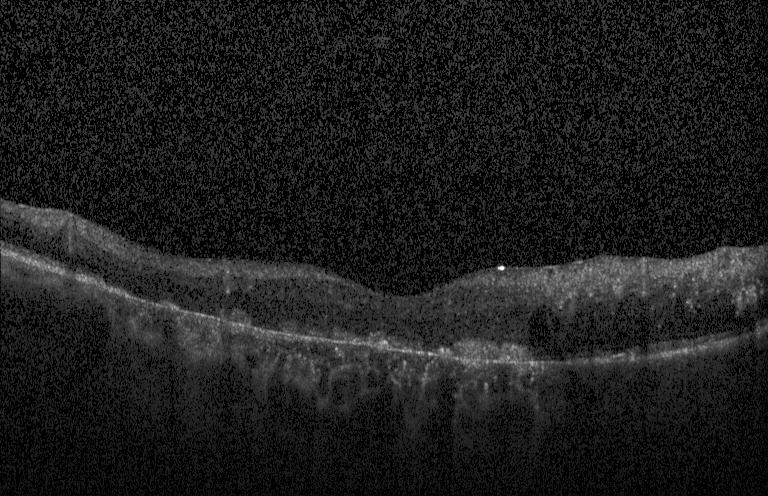
Optical coherence tomography B-scan · acquired on a Heidelberg Spectralis · spectral-domain OCT. Impression: choroidal neovascularization (CNV).